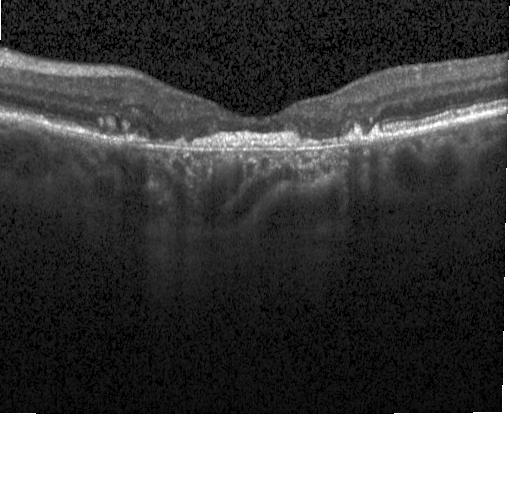

Impression: a choroidal neovascular membrane.